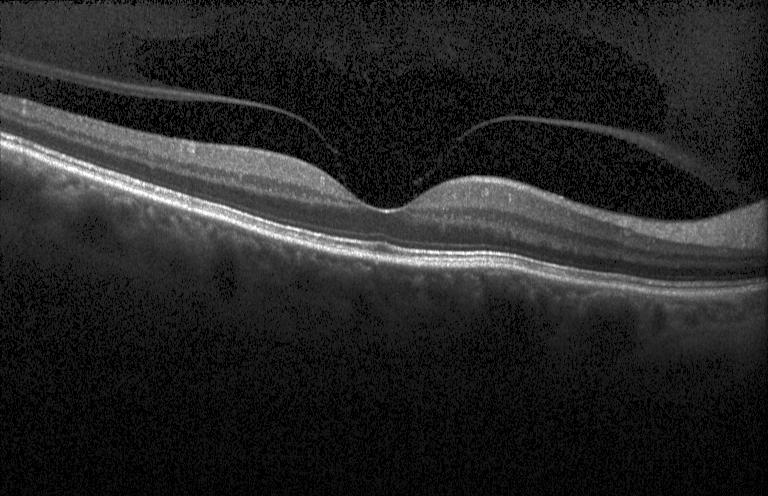 Optical coherence tomography B-scan; centered on the fovea — This B-scan demonstrates neither CNV, DME, nor drusen.